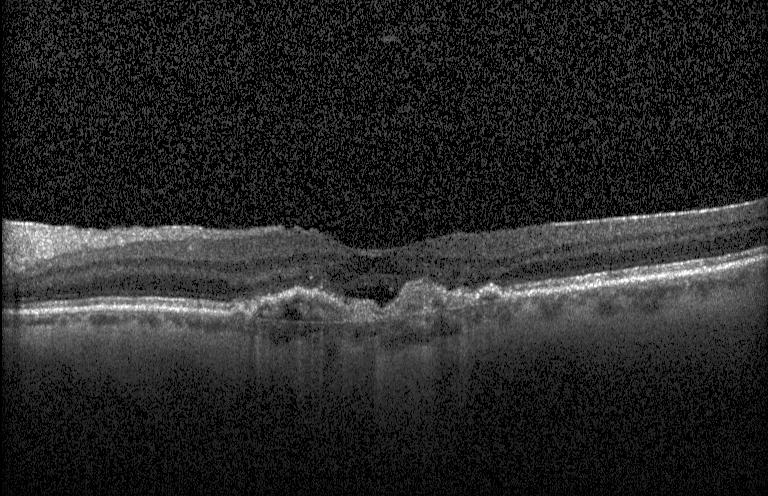 Optical coherence tomography B-scan; spectral-domain optical coherence tomography; fovea-centered.
Choroidal neovascularization (CNV).